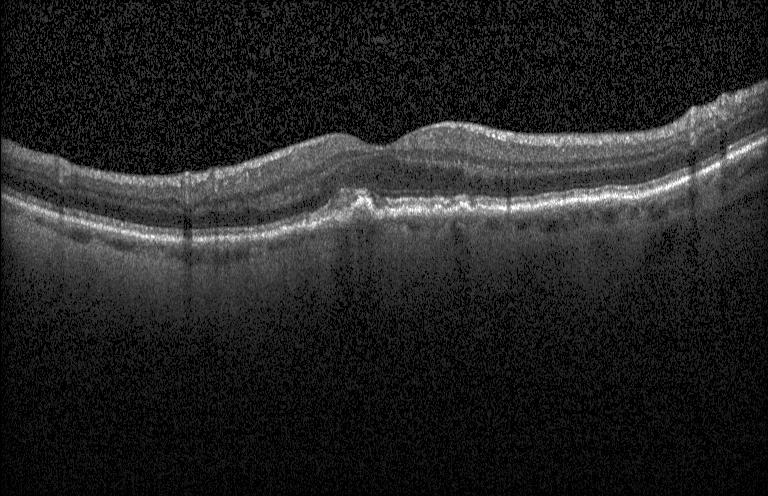 Horizontal scan through the fovea, optical coherence tomography scan — Finding: drusen.